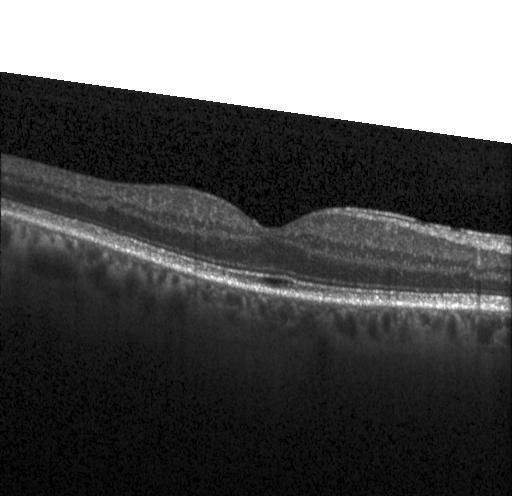

Macular OCT demonstrating no evidence of CNV, DME, or drusen.